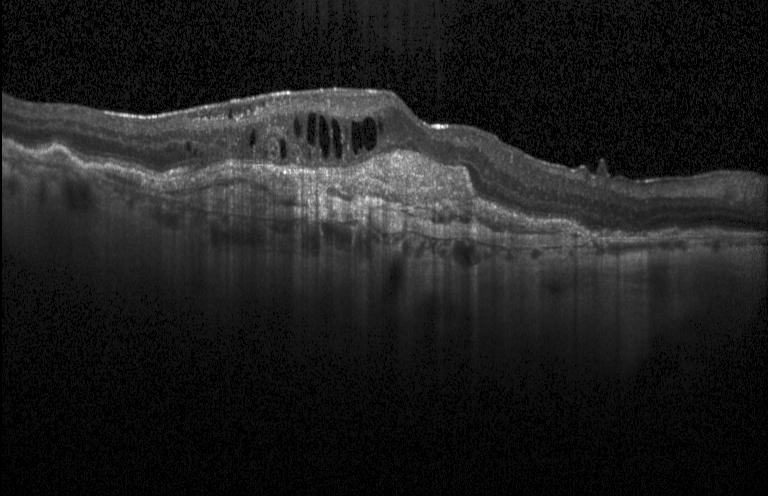 OCT finding: a choroidal neovascular membrane.